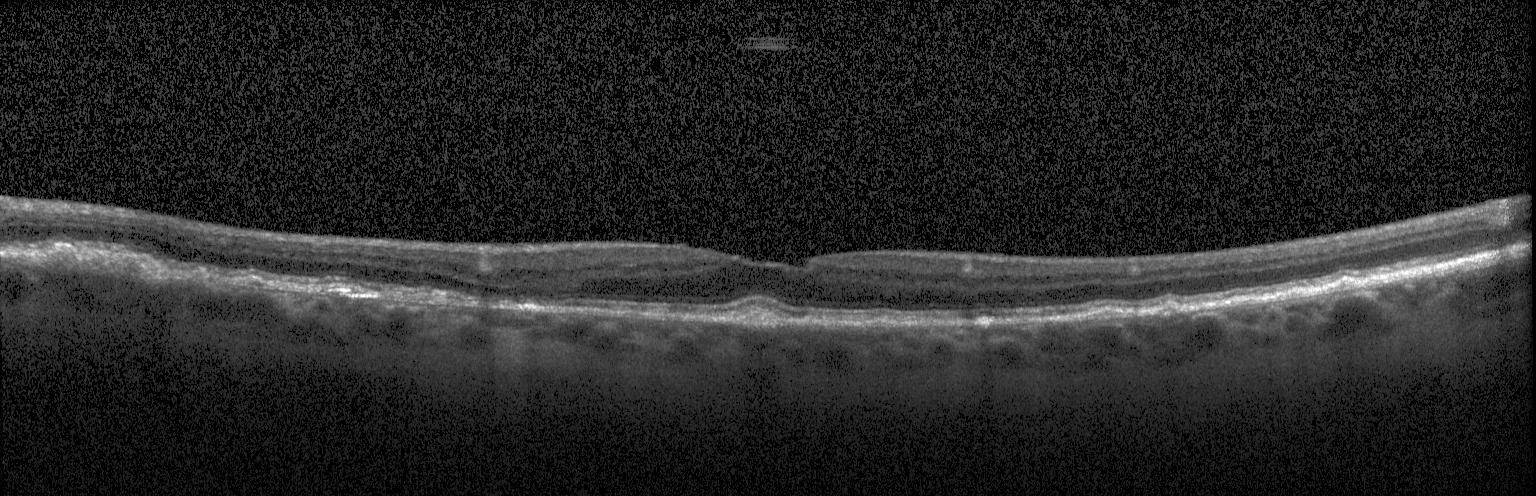
Instrument: Heidelberg Spectralis. Retinal OCT B-scan. Centered on the fovea — OCT finding: drusen.